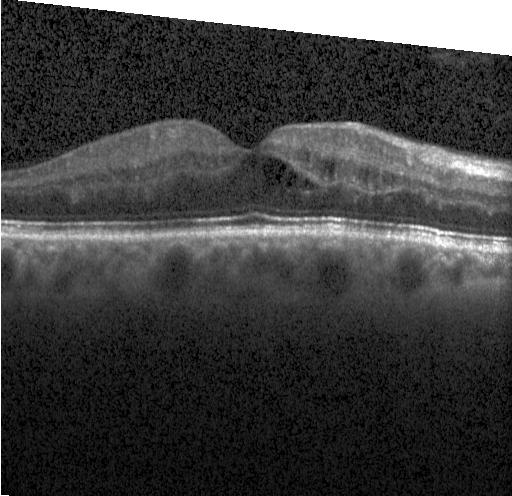 Impression: diabetic macular edema (DME).